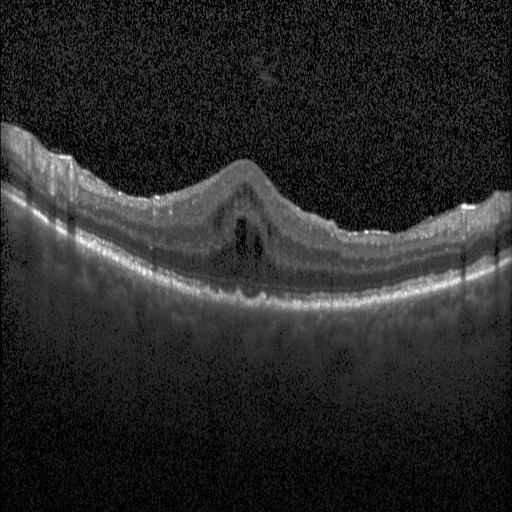

Spectral-domain OCT B-scan: diabetic macular edema.